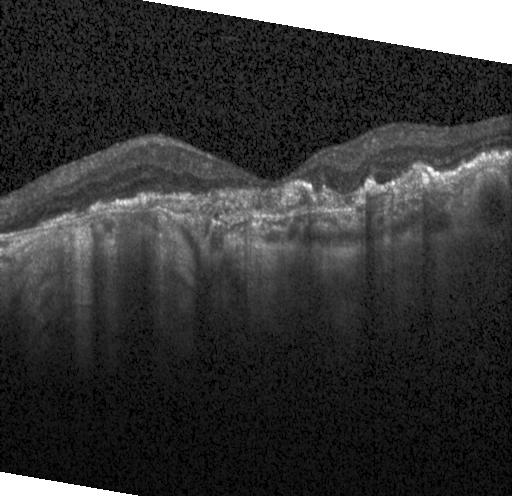

Acquired on a Heidelberg Spectralis · optical coherence tomography scan — Diagnosis: choroidal neovascularization (CNV).